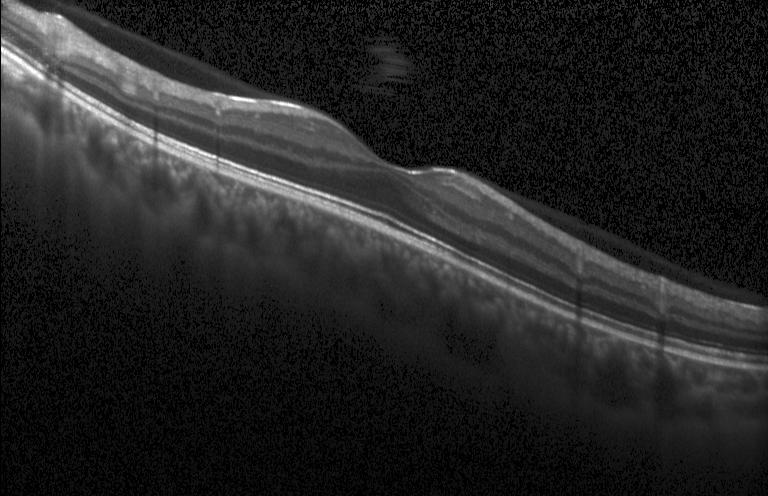

Spectral-domain optical coherence tomography, Heidelberg Spectralis OCT system, retinal OCT B-scan, macular scan. OCT finding: neither CNV, DME, nor drusen.